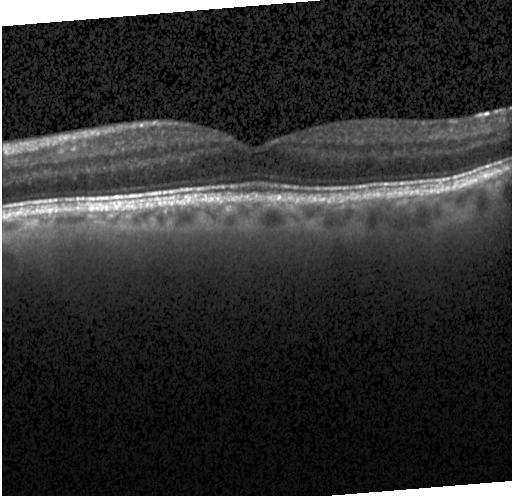

Optical coherence tomography B-scan. Finding: no CNV, no DME, and no drusen.